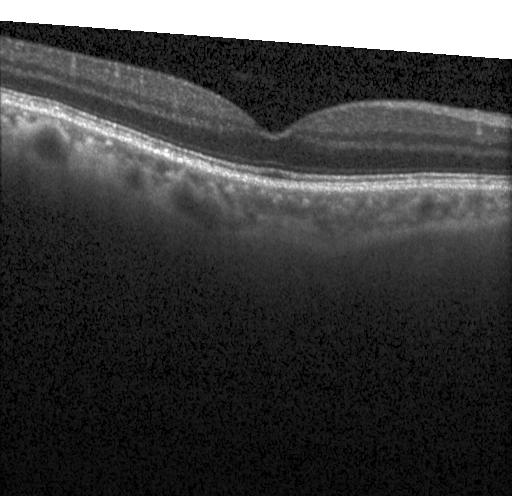

Diagnosis: no evidence of CNV, DME, or drusen.